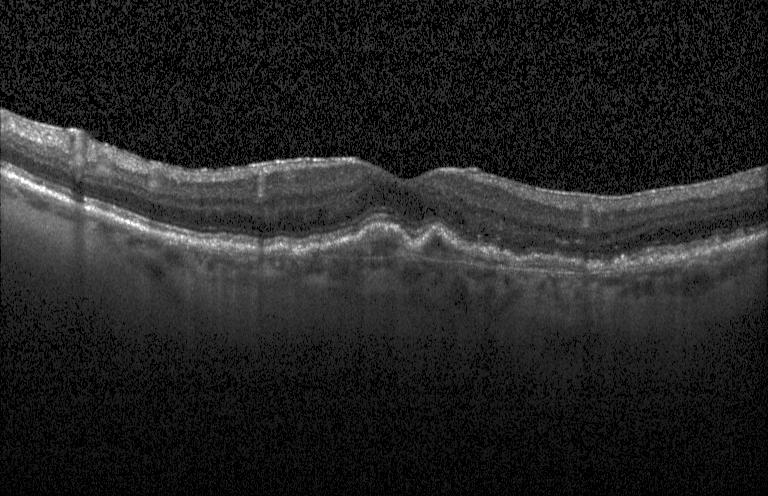 A choroidal neovascular membrane.